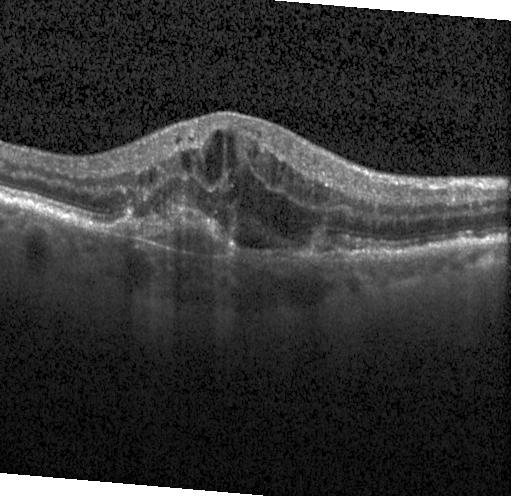
Retinal OCT B-scan, Heidelberg Spectralis, SD-OCT, fovea-centered. Choroidal neovascularization (CNV).